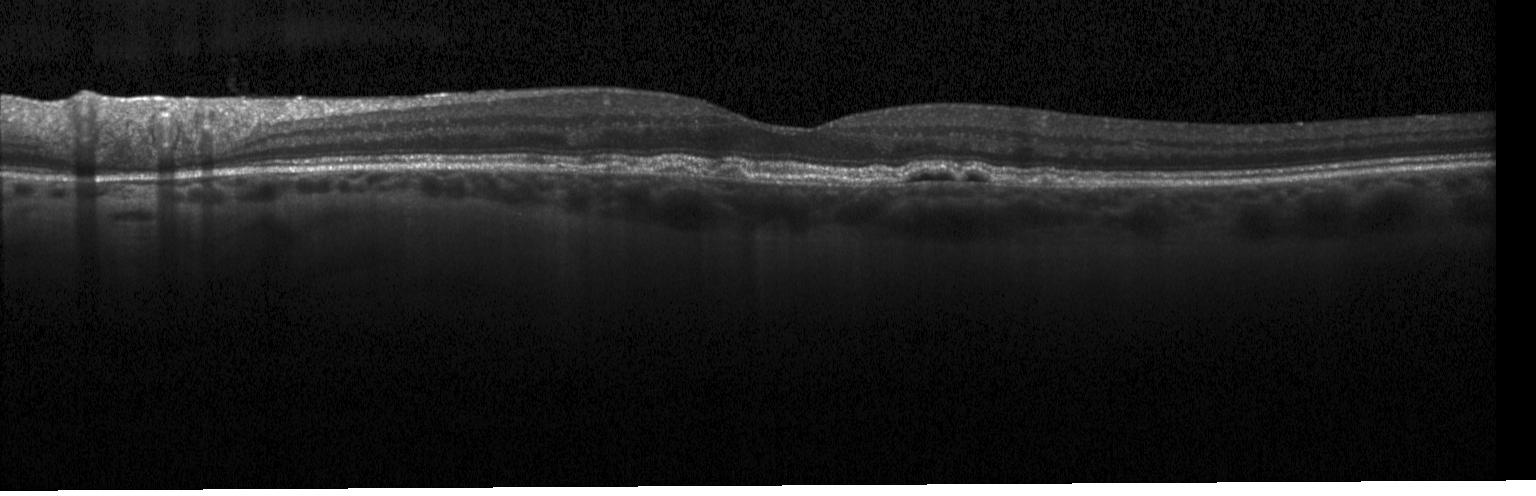
Diagnosis: drusen.